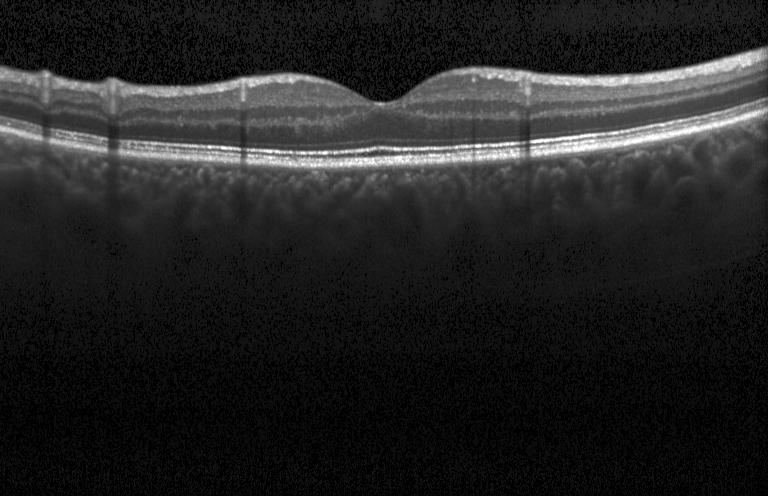

Centered on the fovea · spectral-domain OCT · Heidelberg Spectralis OCT system · OCT line scan. Impression: neither CNV, DME, nor drusen.